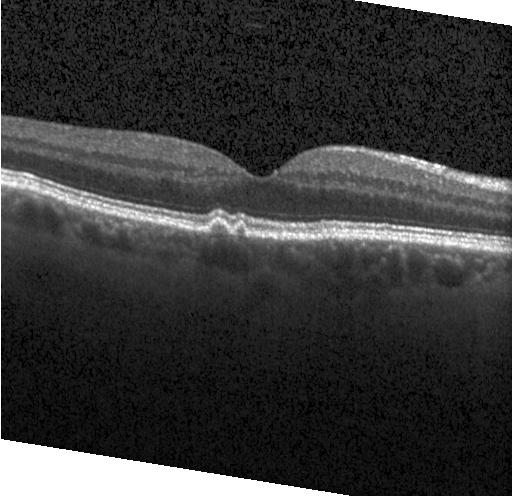
Macular OCT: drusen.